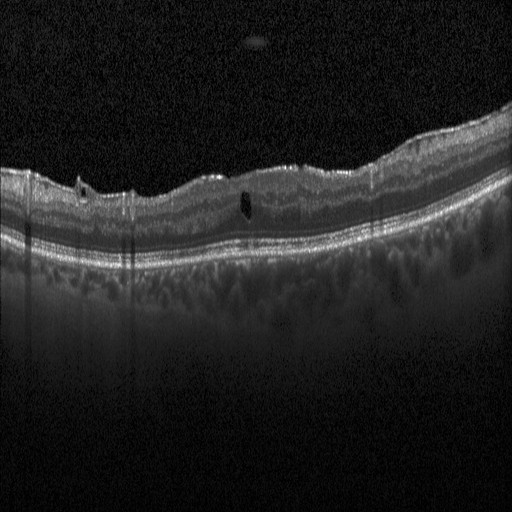

Assessment: DME.